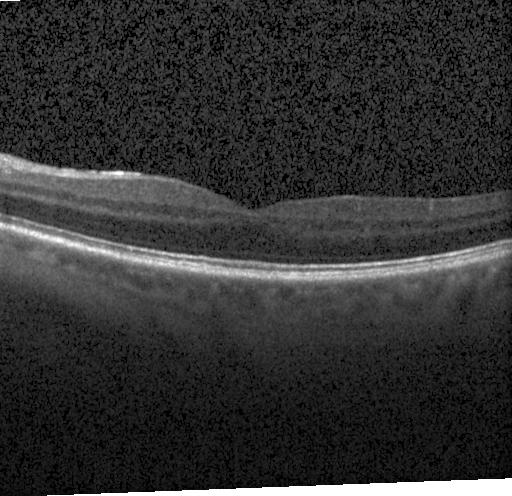
Spectral-domain optical coherence tomography. Retinal OCT cross-section. Instrument: Heidelberg Spectralis
Impression: no evidence of choroidal neovascularization, diabetic macular edema, or drusen.